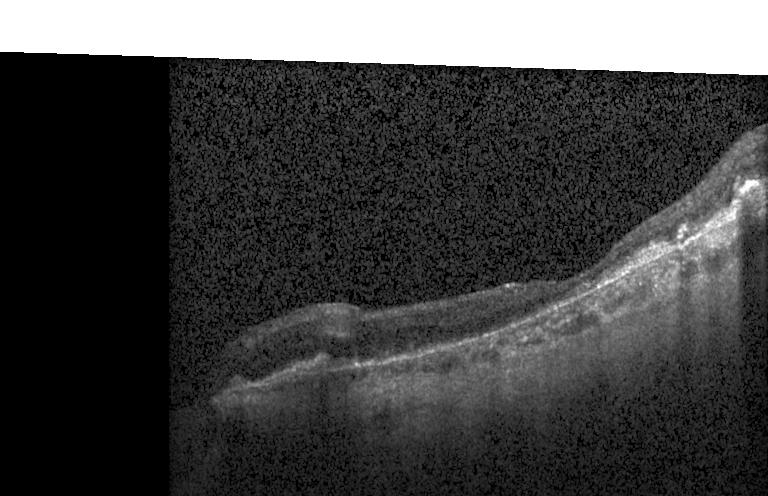 Retinal OCT B-scan. OCT finding: choroidal neovascularization.